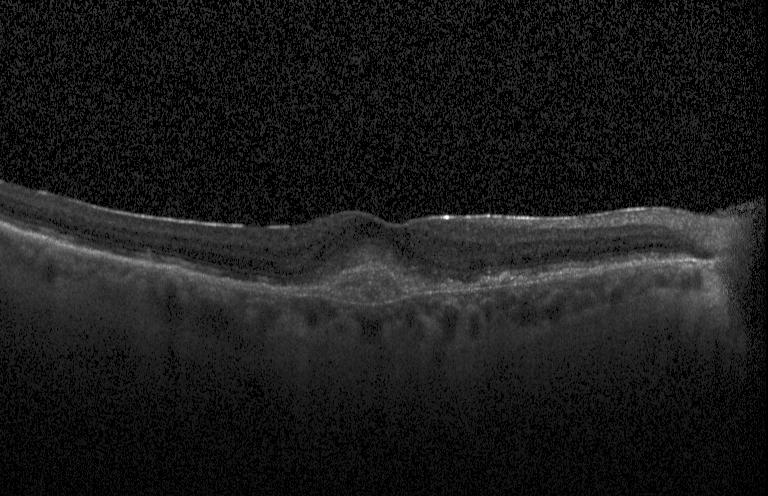 OCT line scan. OCT finding: a choroidal neovascular membrane.